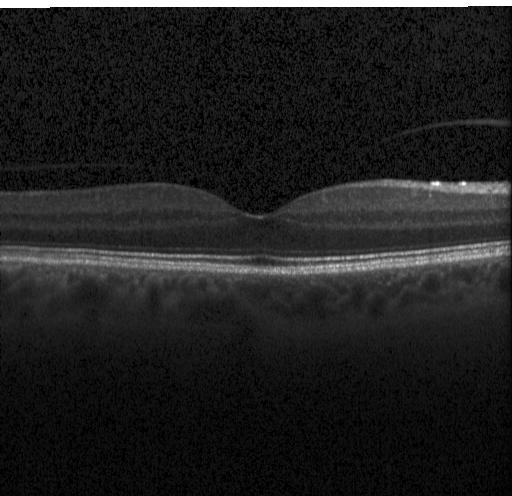
OCT B-scan; instrument: Heidelberg Spectralis; spectral-domain OCT; macular scan — Finding: no choroidal neovascularization, diabetic macular edema, or drusen.